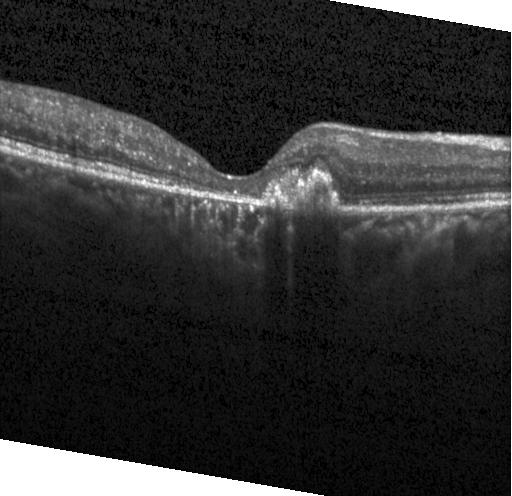 OCT line scan — Impression: choroidal neovascularization.